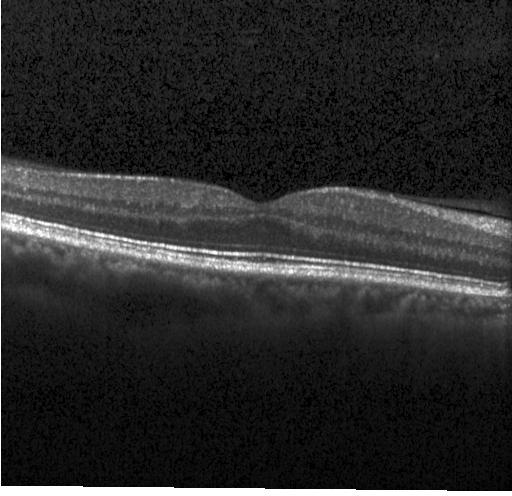
Instrument: Heidelberg Spectralis, retinal OCT B-scan, fovea-centered, SD-OCT
Diagnosis: neither choroidal neovascularization, diabetic macular edema, nor drusen.